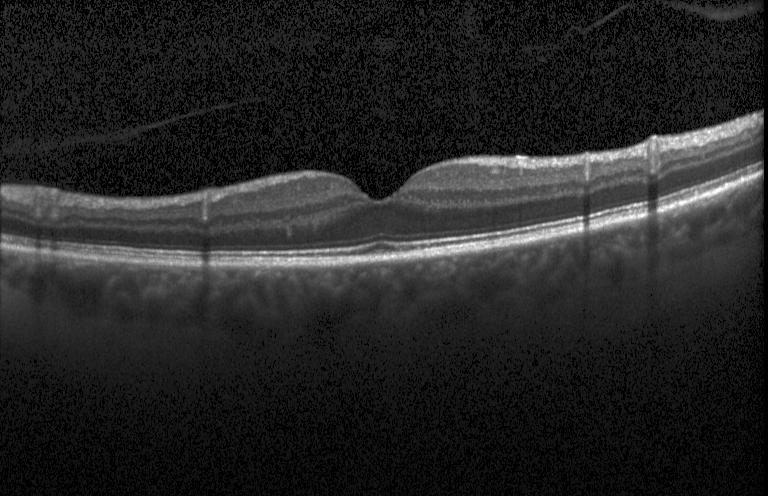
SD-OCT, macular scan, retinal OCT cross-section. Macular OCT: no CNV, no DME, and no drusen.